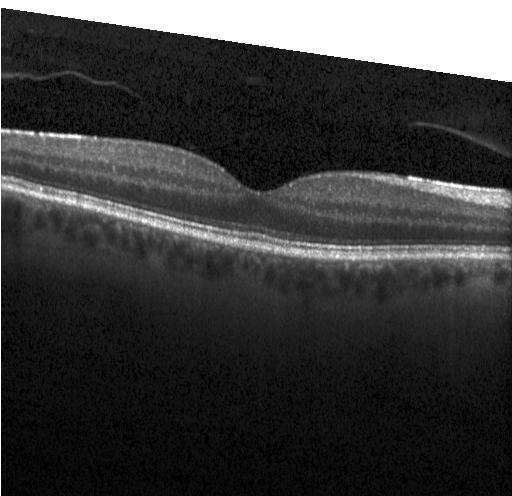
OCT B-scan showing no CNV, DME, or drusen.